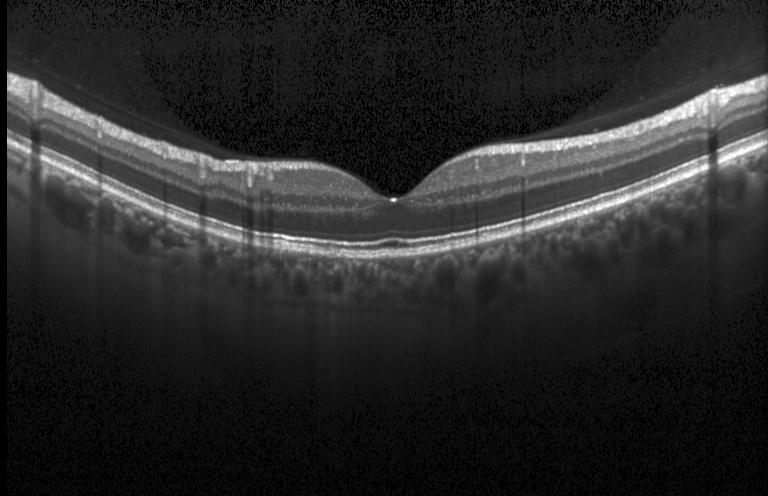 Retinal OCT B-scan; fovea-centered. No choroidal neovascularization, diabetic macular edema, or drusen.